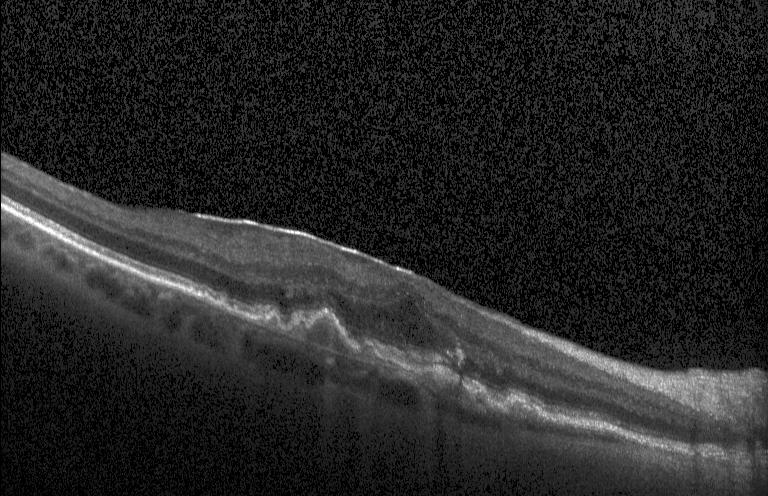

Macular OCT demonstrating sub-RPE drusenoid deposits.